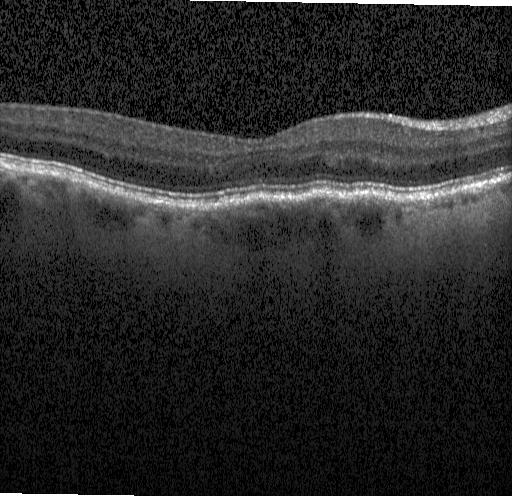 OCT line scan — Diagnosis: no evidence of choroidal neovascularization, diabetic macular edema, or drusen.